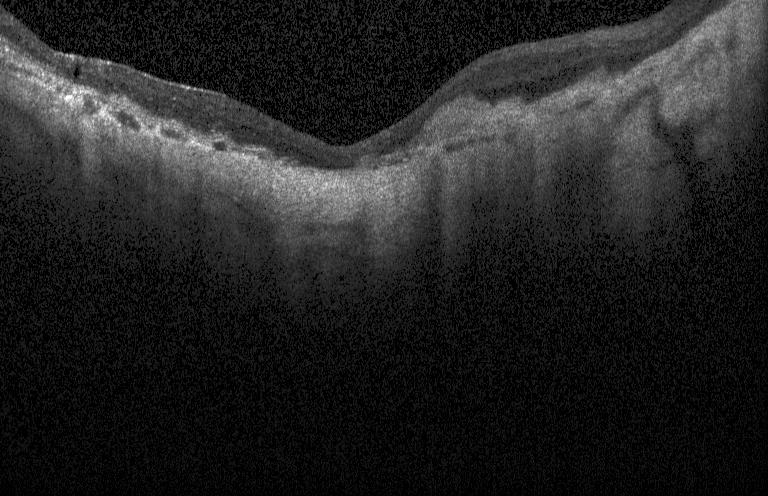 Dx: choroidal neovascularization (CNV).